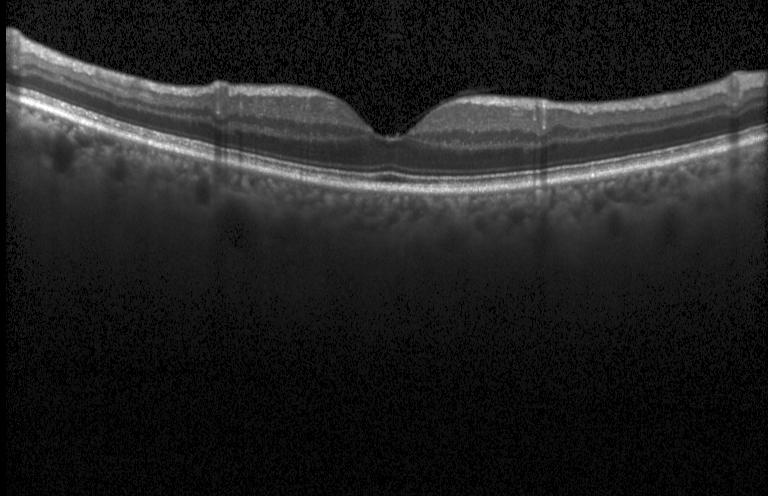

Heidelberg Spectralis; horizontal scan through the fovea; optical coherence tomography scan; spectral-domain OCT. OCT finding: no CNV, DME, or drusen.